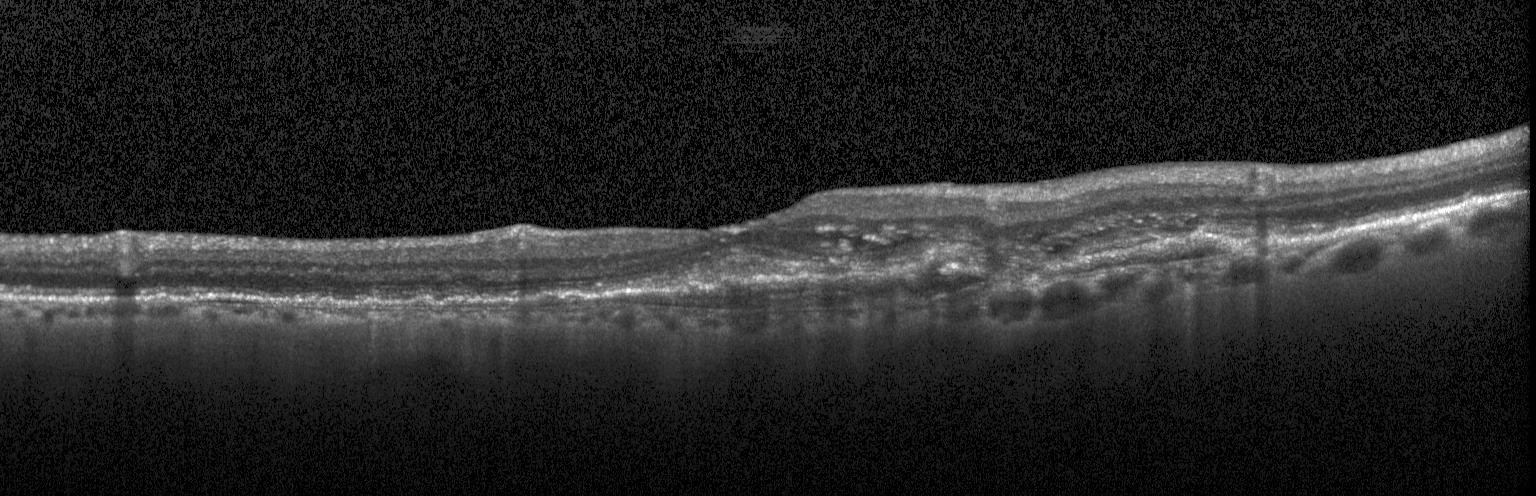

SD-OCT; optical coherence tomography B-scan; through the macula.
Assessment: CNV.